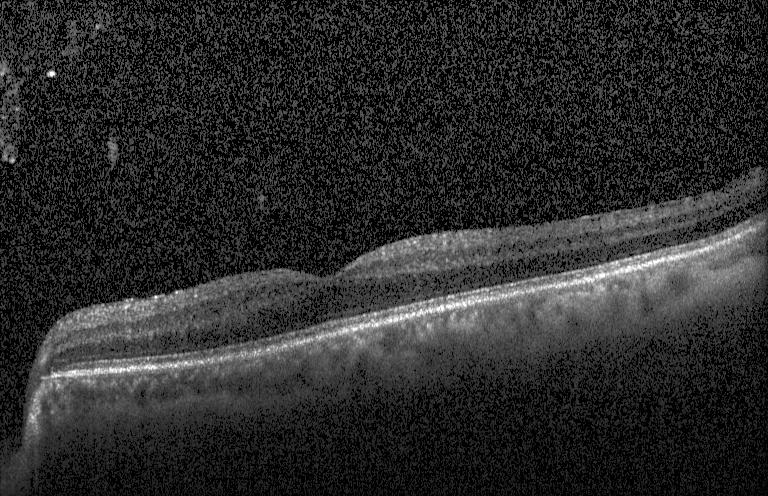
Fovea-centered · spectral-domain OCT · optical coherence tomography scan · instrument: Heidelberg Spectralis
Impression: no choroidal neovascularization, no diabetic macular edema, and no drusen.